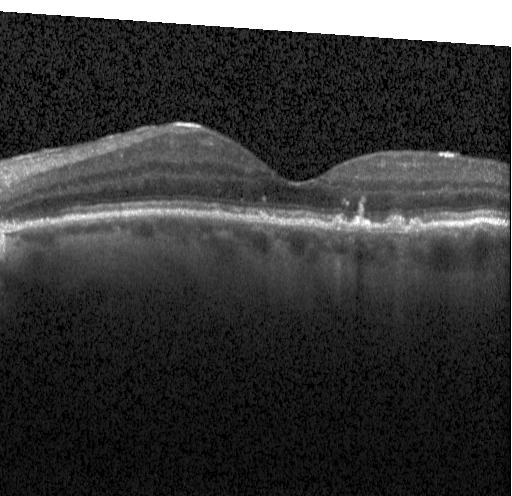 OCT B-scan · fovea-centered · acquired on a Heidelberg Spectralis · spectral-domain OCT.
Diagnosis: sub-RPE drusenoid deposits.